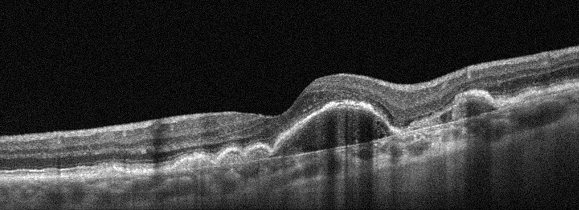
Optical coherence tomography scan; left eye; macular scan
The scan shows AMD.